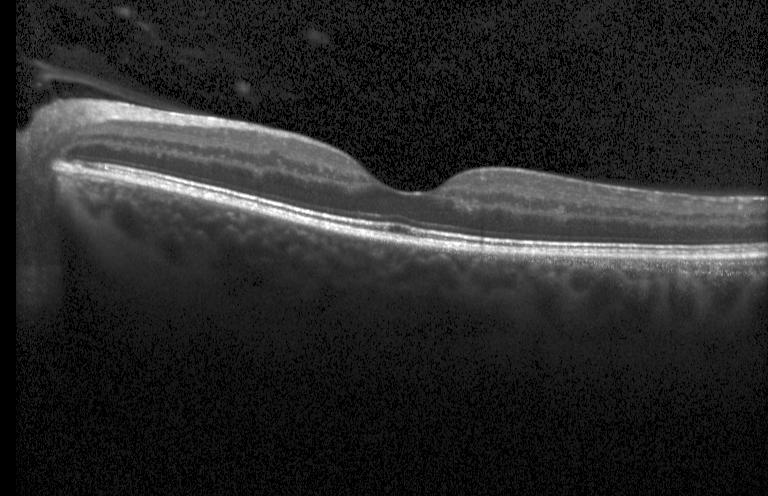

Retinal OCT cross-section, spectral-domain optical coherence tomography, Heidelberg Spectralis OCT system — Diagnosis: no evidence of choroidal neovascularization, diabetic macular edema, or drusen.